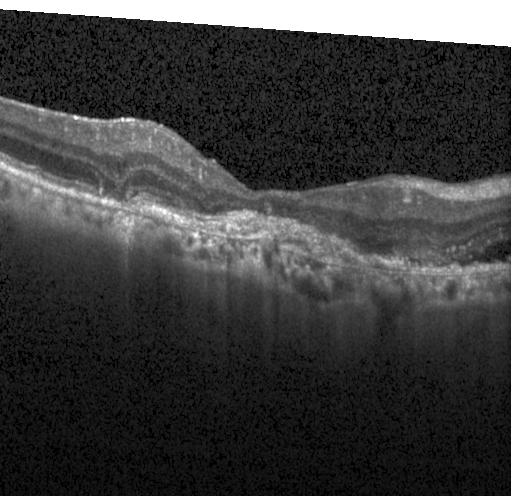
Spectral-domain OCT · acquired on a Heidelberg Spectralis · optical coherence tomography scan. The scan shows choroidal neovascularization.